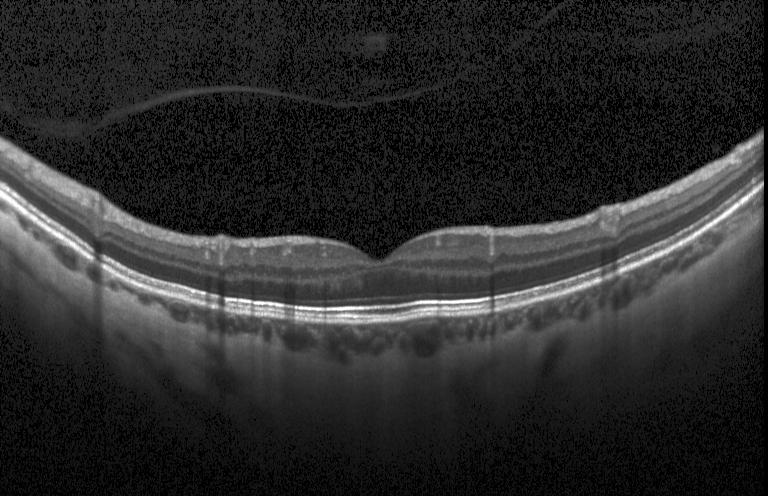

Finding: neither choroidal neovascularization, diabetic macular edema, nor drusen.